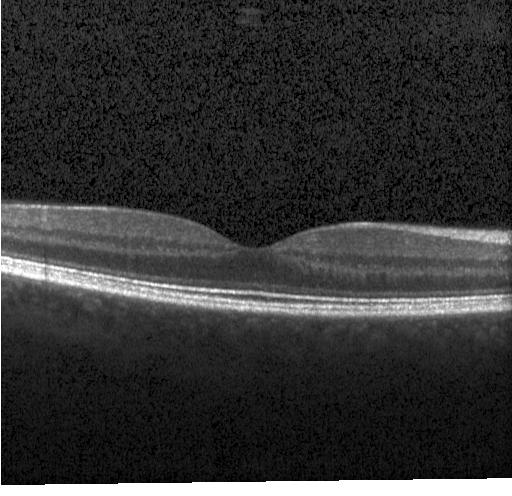

Impression: no evidence of choroidal neovascularization, diabetic macular edema, or drusen.